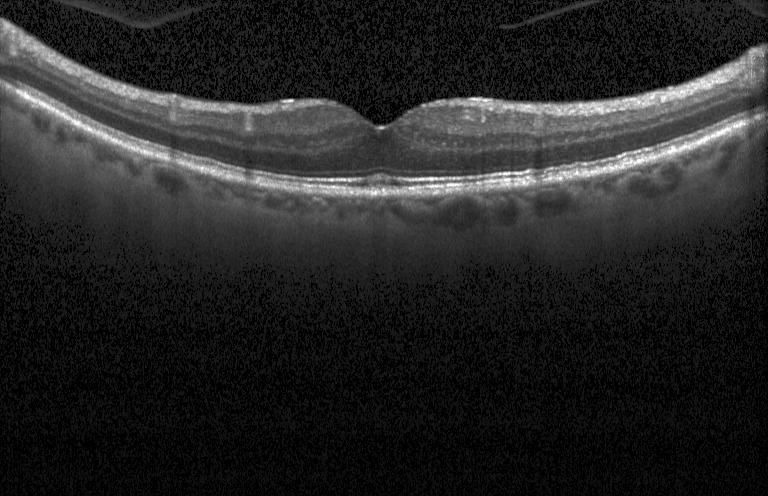

Heidelberg Spectralis; retinal OCT B-scan; spectral-domain OCT — Finding: no choroidal neovascularization, no diabetic macular edema, and no drusen.